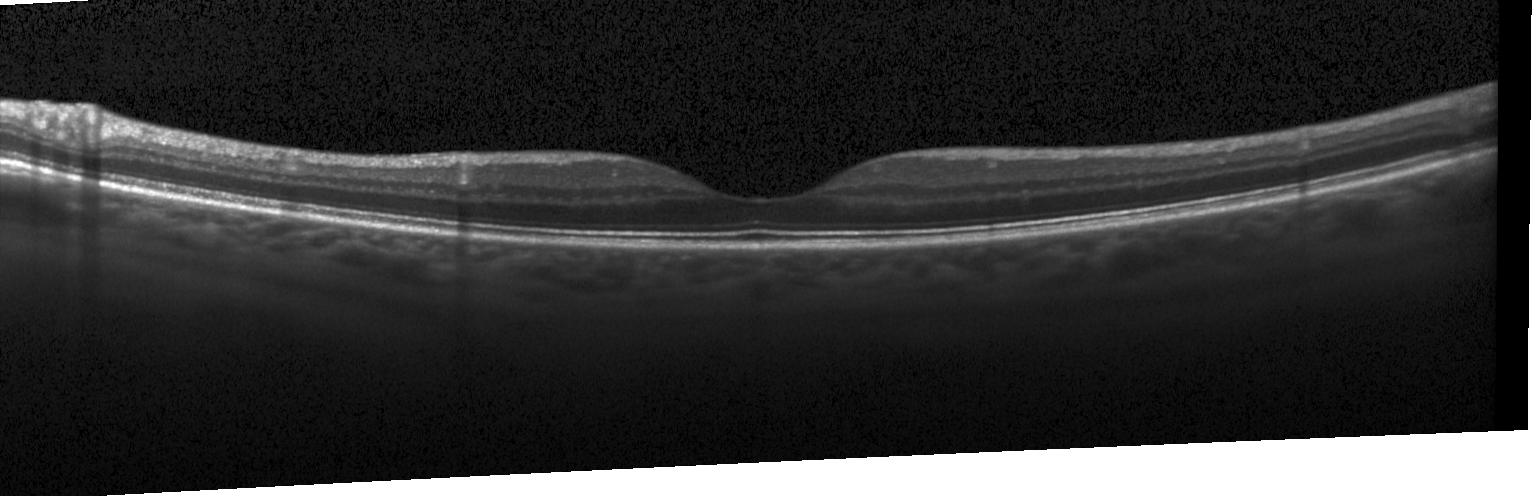

Through the macula, spectral-domain OCT, optical coherence tomography B-scan — Macular OCT: no choroidal neovascularization, no diabetic macular edema, and no drusen.